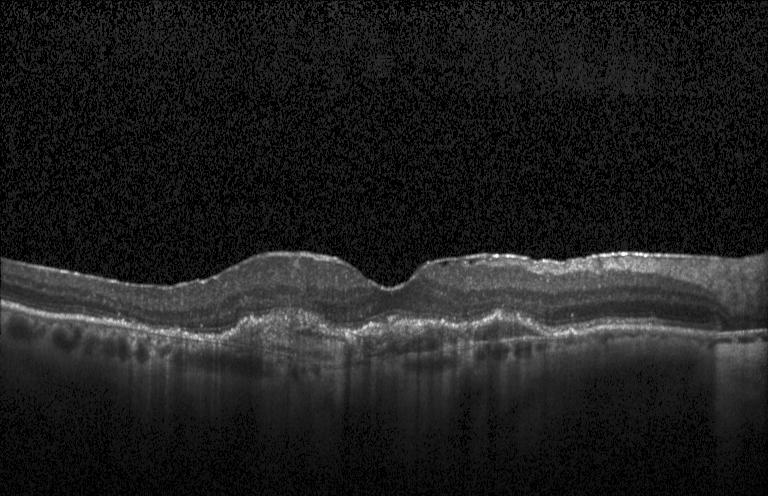 Optical coherence tomography scan. Choroidal neovascularization.